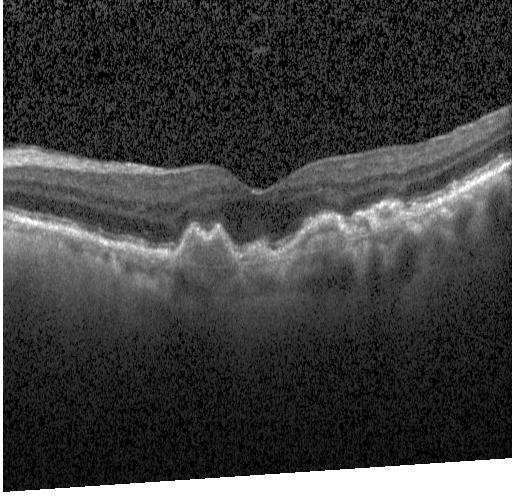 Retinal OCT cross-section.
Dx: a choroidal neovascular membrane.